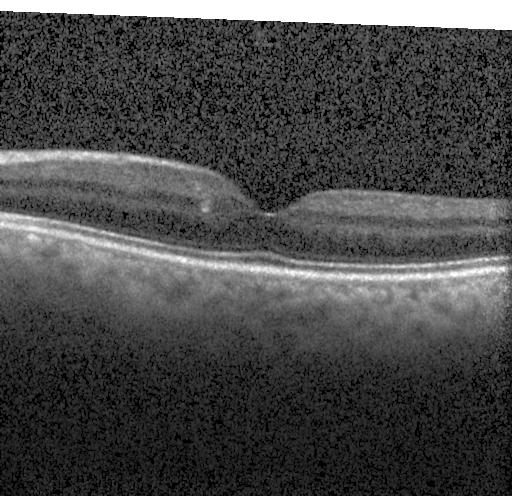 OCT B-scan. Spectral-domain OCT. Macular scan — The scan shows no choroidal neovascularization, no diabetic macular edema, and no drusen.